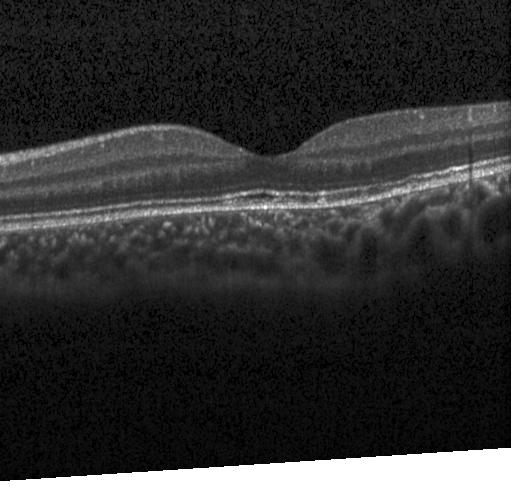
Spectral-domain OCT, retinal OCT cross-section. Assessment: no choroidal neovascularization, no diabetic macular edema, and no drusen.